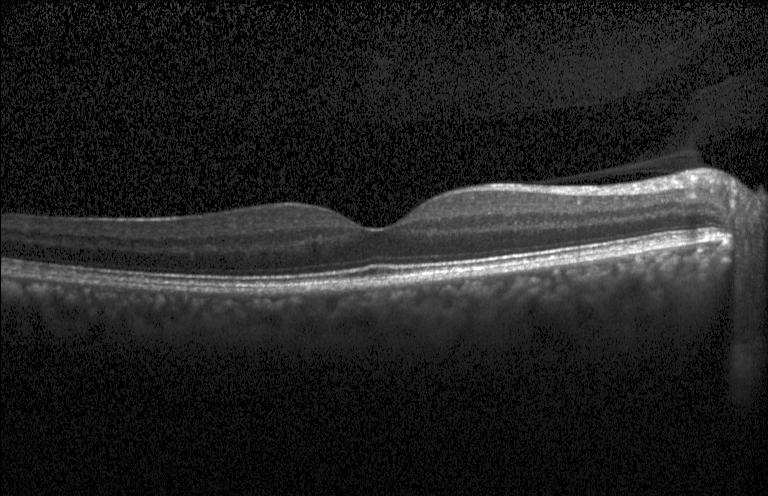
Centered on the fovea, Heidelberg Spectralis OCT system, retinal OCT cross-section. This B-scan demonstrates no evidence of choroidal neovascularization, diabetic macular edema, or drusen.